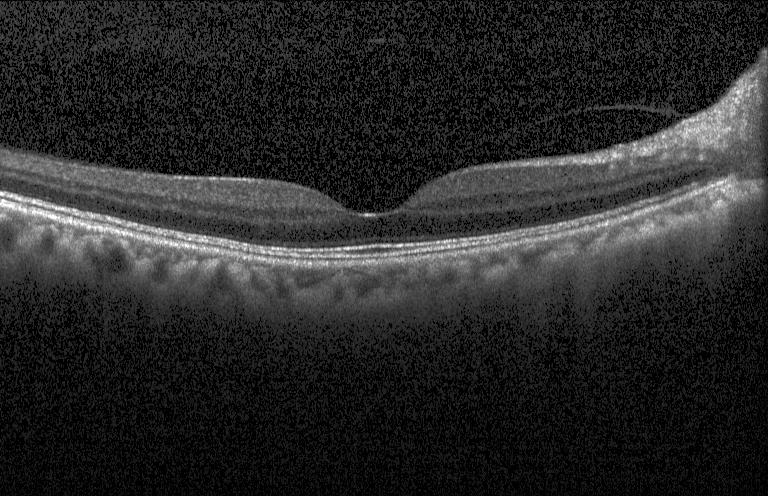 Spectral-domain optical coherence tomography. Retinal OCT B-scan. Heidelberg Spectralis — This B-scan demonstrates no CNV, DME, or drusen.